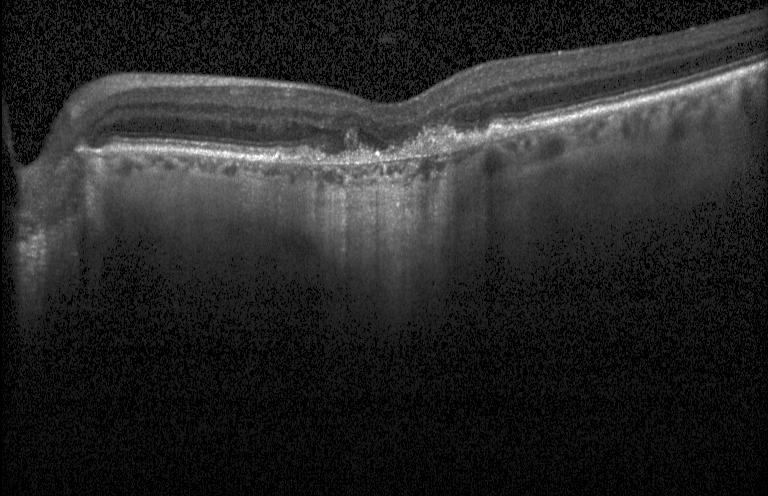 Macular OCT demonstrating a choroidal neovascular membrane.